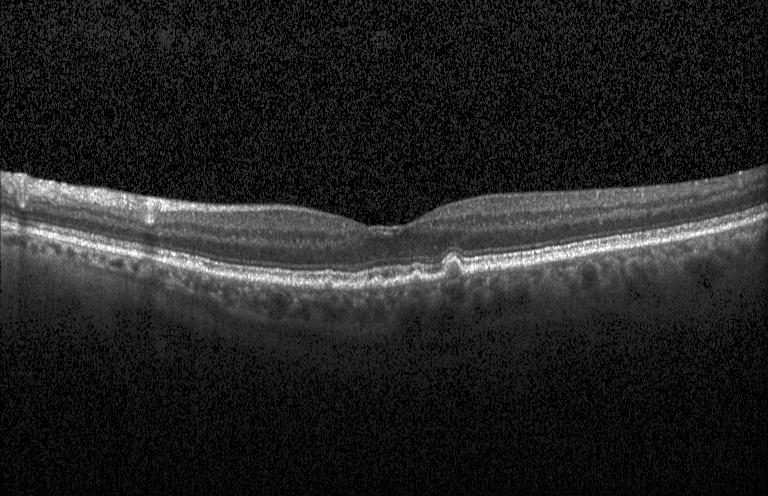
Finding: multiple drusen.